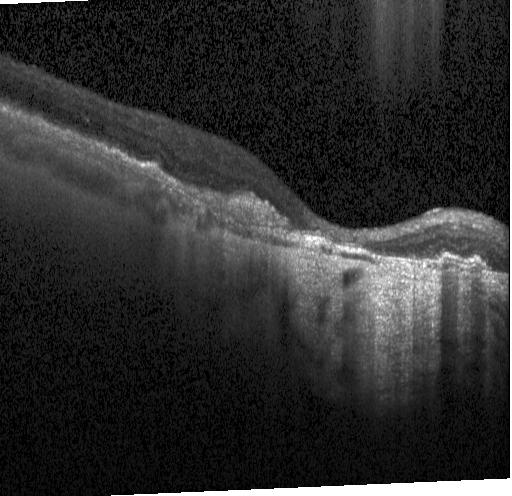 Diagnosis: a choroidal neovascular membrane.